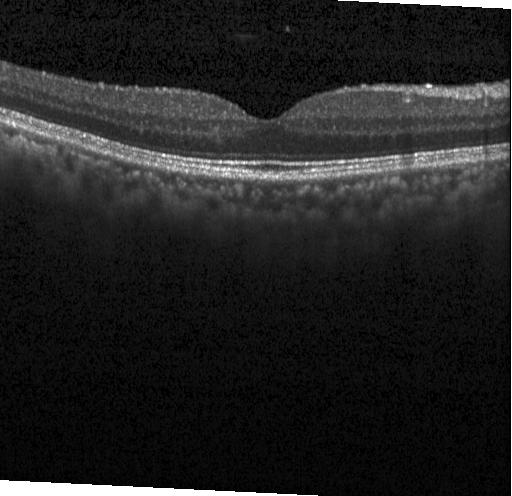 OCT line scan, acquired on a Heidelberg Spectralis, spectral-domain optical coherence tomography, through the macula
Dx: no choroidal neovascularization, diabetic macular edema, or drusen.